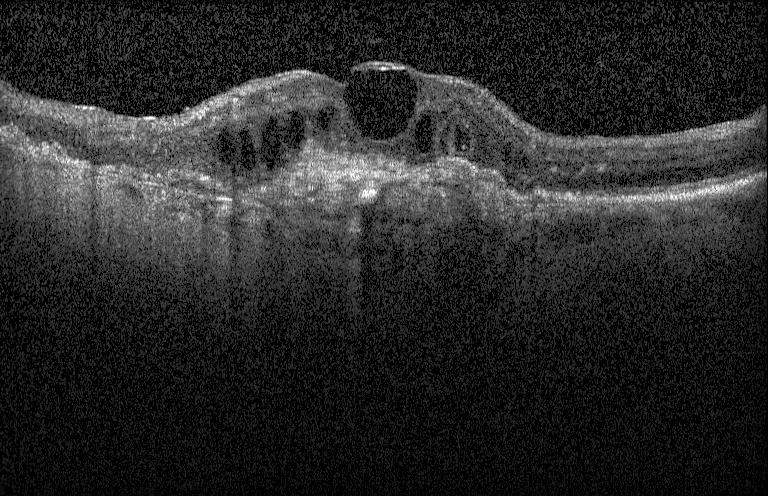
Retinal OCT B-scan — OCT finding: choroidal neovascularization.